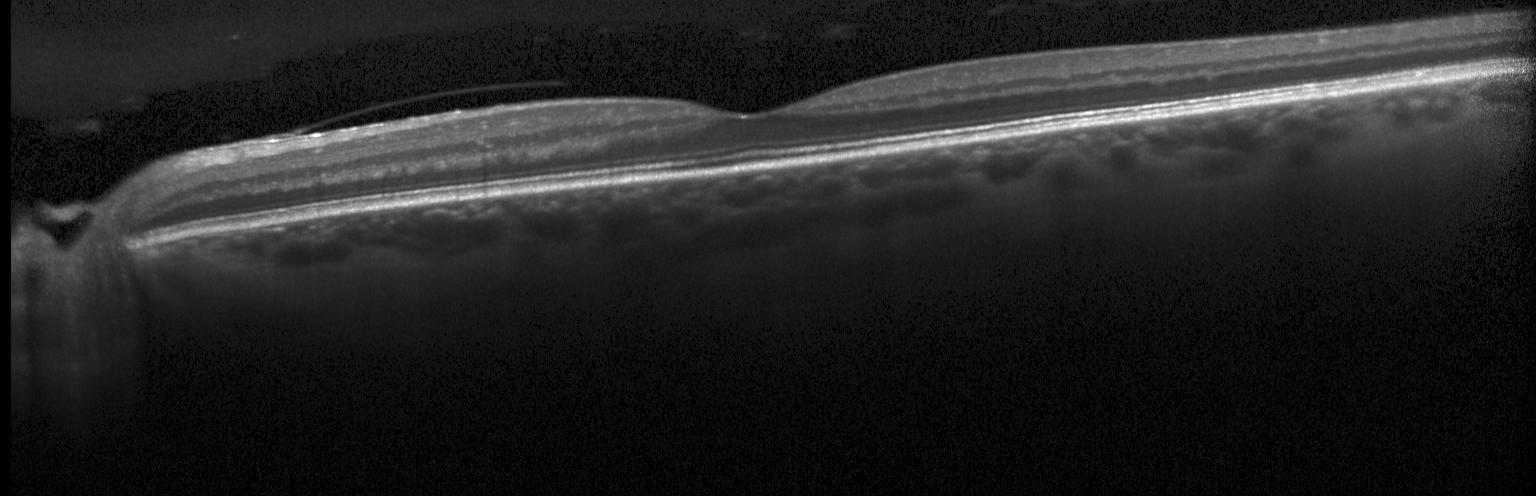
Dx: no evidence of choroidal neovascularization, diabetic macular edema, or drusen.